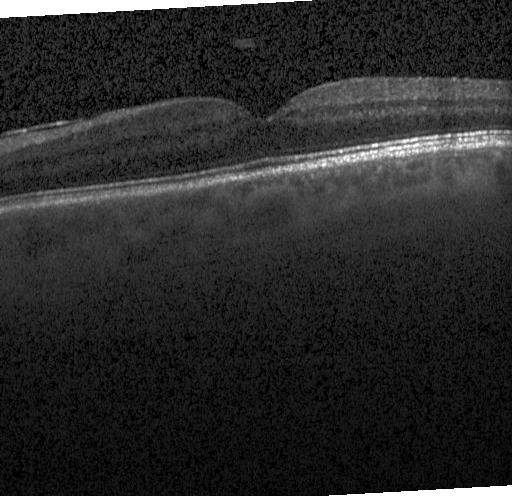

Finding: no choroidal neovascularization, no diabetic macular edema, and no drusen.